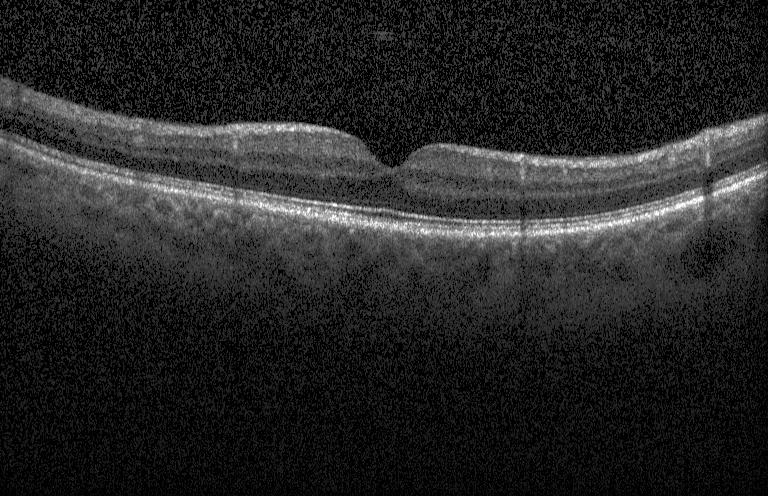

Retinal OCT B-scan; spectral-domain optical coherence tomography. This B-scan demonstrates no choroidal neovascularization, no diabetic macular edema, and no drusen.